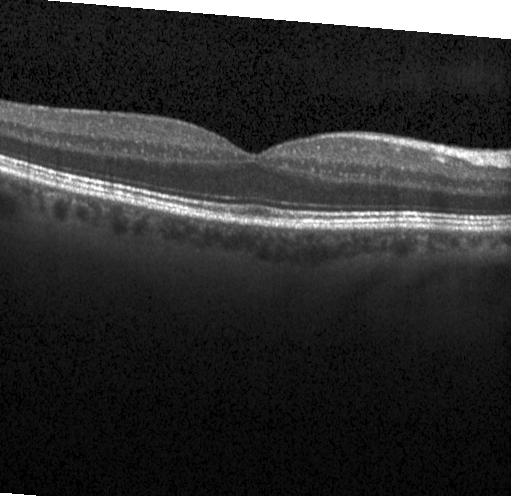
Finding: no evidence of choroidal neovascularization, diabetic macular edema, or drusen.